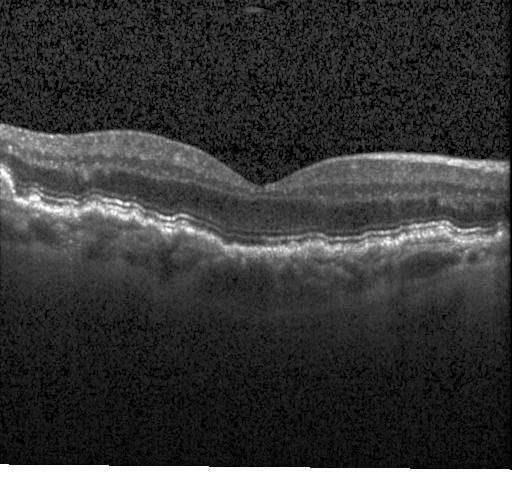
Instrument: Heidelberg Spectralis, OCT line scan, SD-OCT.
Diagnosis: drusen.